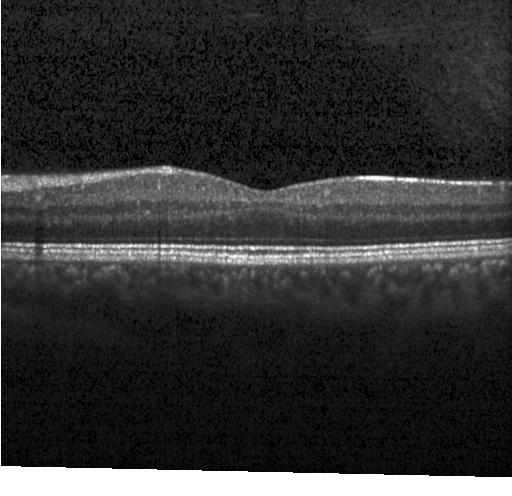 Spectral-domain OCT B-scan: neither CNV, DME, nor drusen.